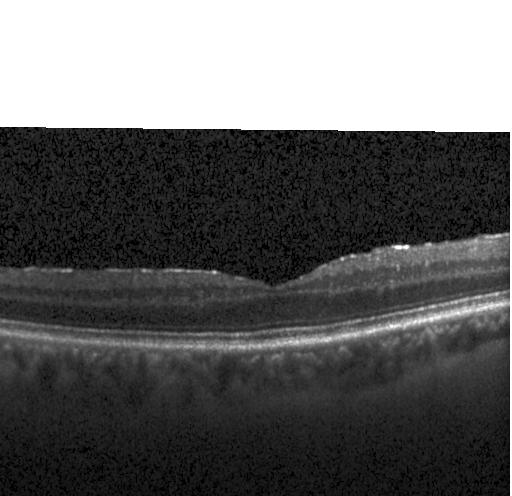
Retinal OCT B-scan.
Assessment: neither choroidal neovascularization, diabetic macular edema, nor drusen.